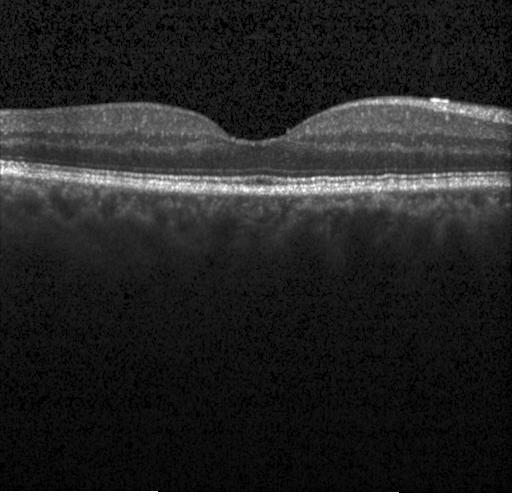 Finding: neither CNV, DME, nor drusen.